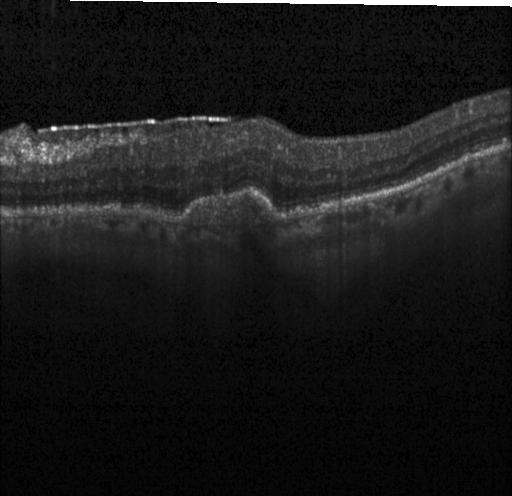 Macular OCT demonstrating choroidal neovascularization (CNV).